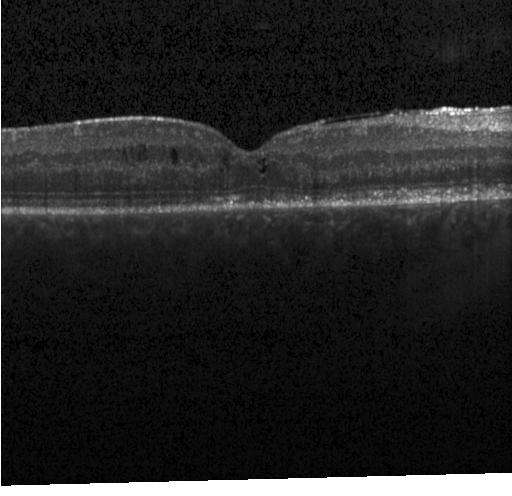
Heidelberg Spectralis · through the macula · retinal OCT cross-section.
Finding: DME.